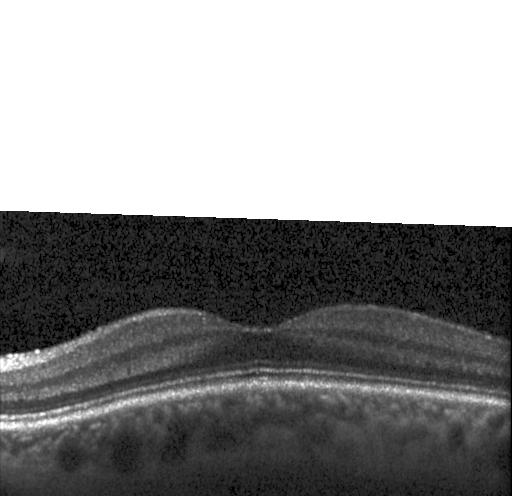

OCT line scan — Macular OCT: no choroidal neovascularization, no diabetic macular edema, and no drusen.